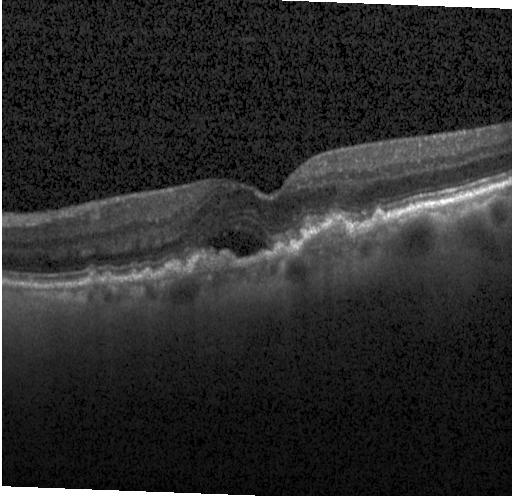
Assessment: a choroidal neovascular membrane.